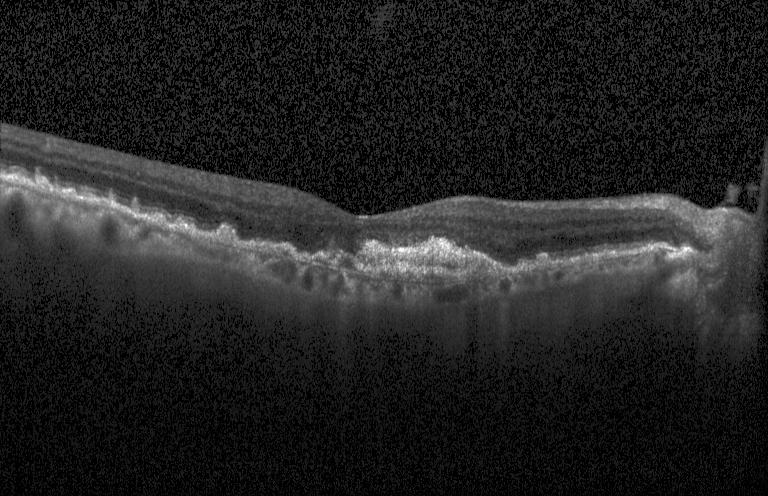

Spectral-domain optical coherence tomography, retinal OCT cross-section, macular scan, Heidelberg Spectralis OCT system. Diagnosis: choroidal neovascularization (CNV).